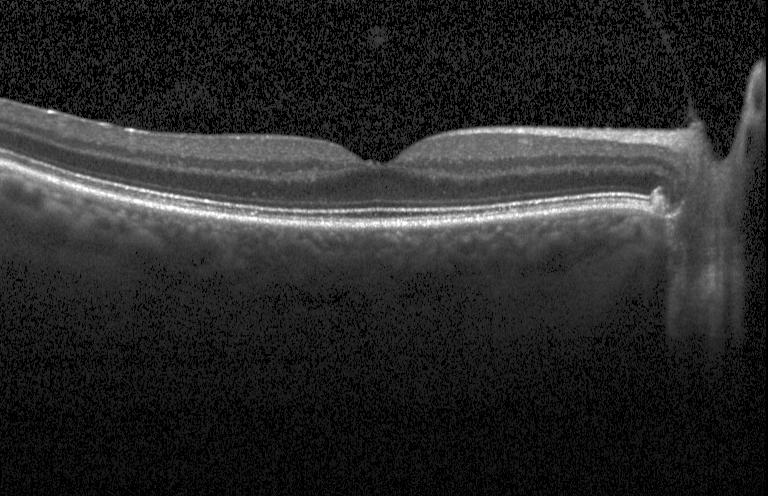
Finding: no evidence of choroidal neovascularization, diabetic macular edema, or drusen.